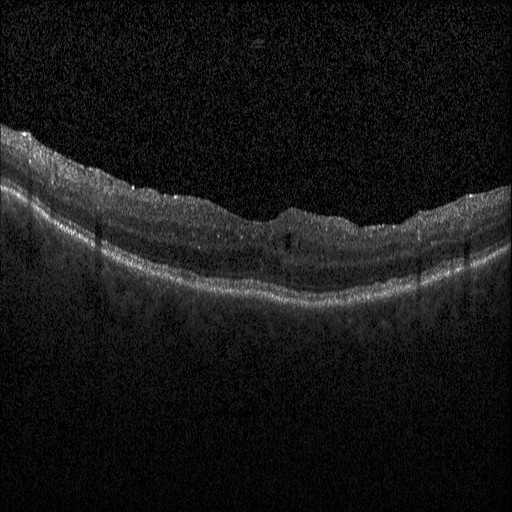

Macular scan; OCT line scan; Heidelberg Spectralis.
Macular OCT: diabetic macular edema (DME).